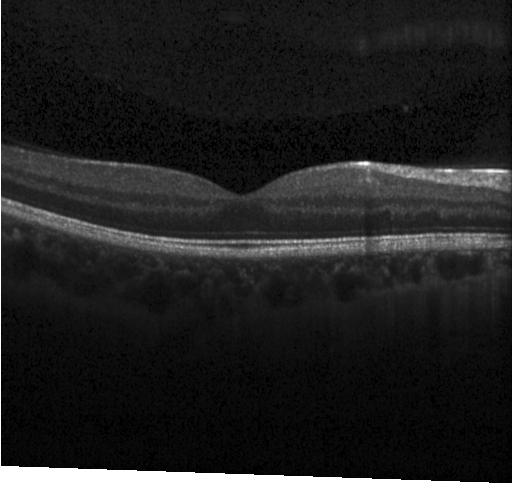 OCT finding: no choroidal neovascularization, diabetic macular edema, or drusen.